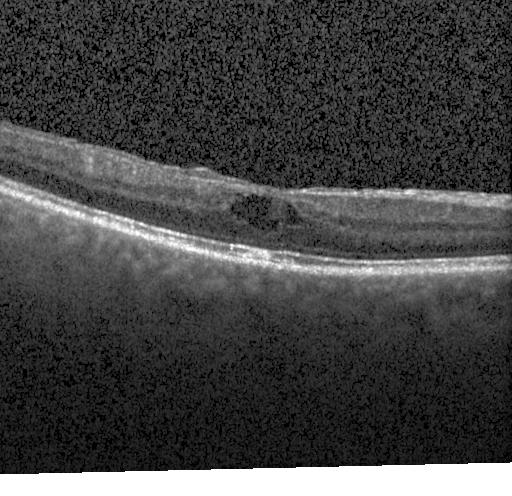

Finding: diabetic macular edema.